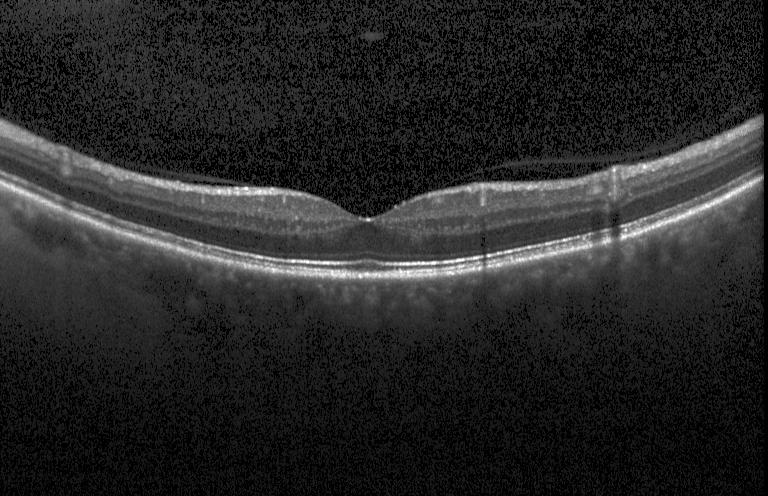

Optical coherence tomography scan; Heidelberg Spectralis OCT system; spectral-domain OCT; centered on the fovea.
Diagnosis: neither CNV, DME, nor drusen.